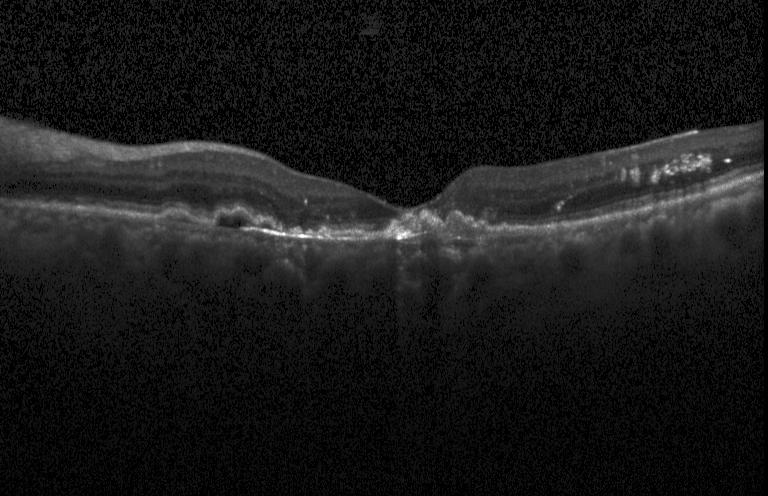 Retinal OCT B-scan · Heidelberg Spectralis OCT system — Impression: a choroidal neovascular membrane.